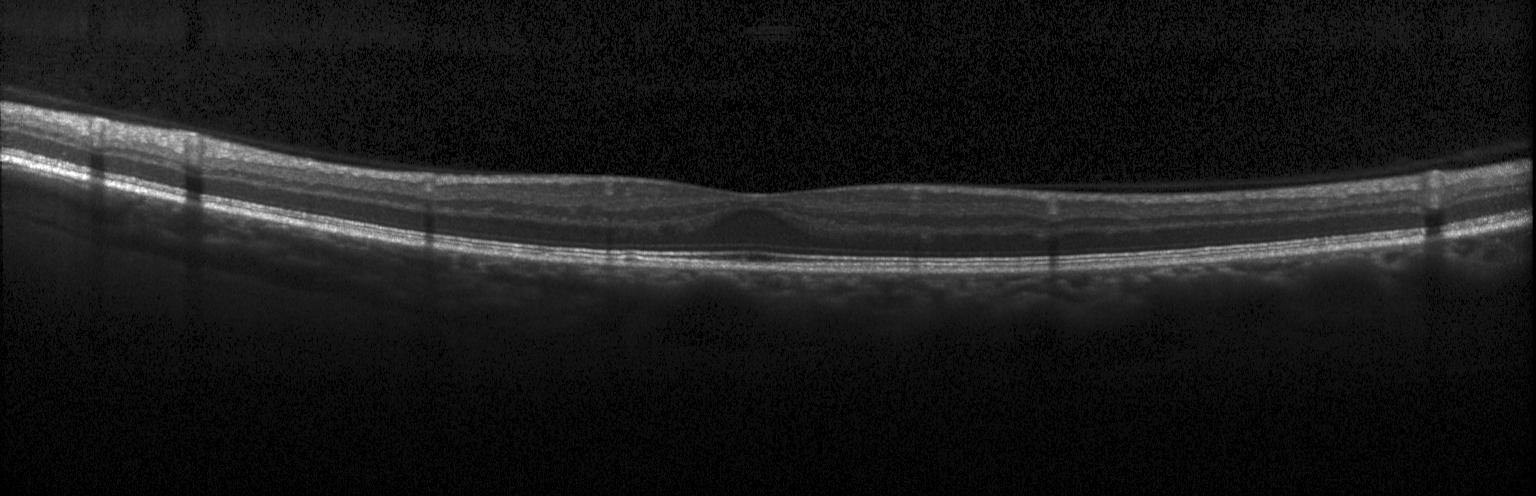

Macular OCT: no choroidal neovascularization, diabetic macular edema, or drusen.